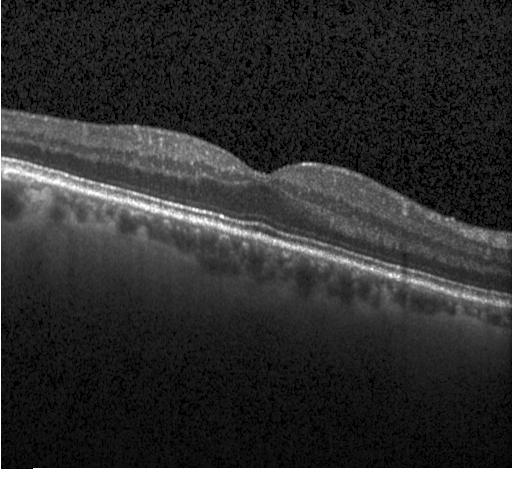
Spectral-domain OCT. Optical coherence tomography scan. Instrument: Heidelberg Spectralis. Finding: neither CNV, DME, nor drusen.